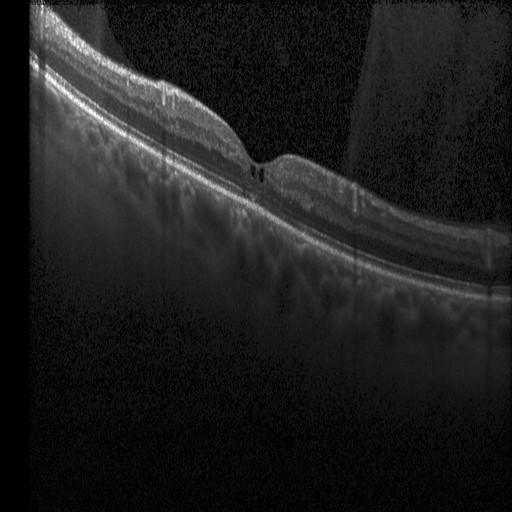 OCT B-scan; centered on the fovea; SD-OCT — Macular OCT: diabetic macular edema (DME).